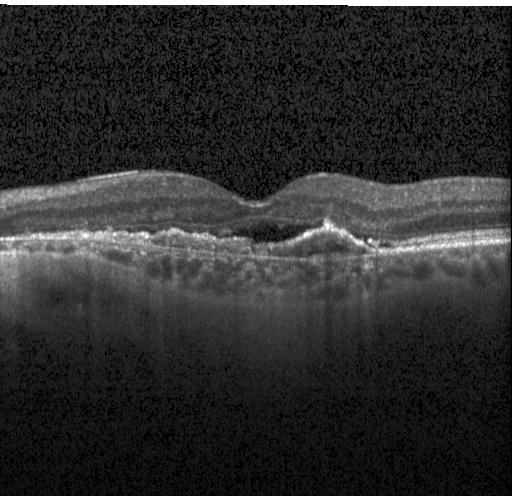 Finding: a choroidal neovascular membrane.